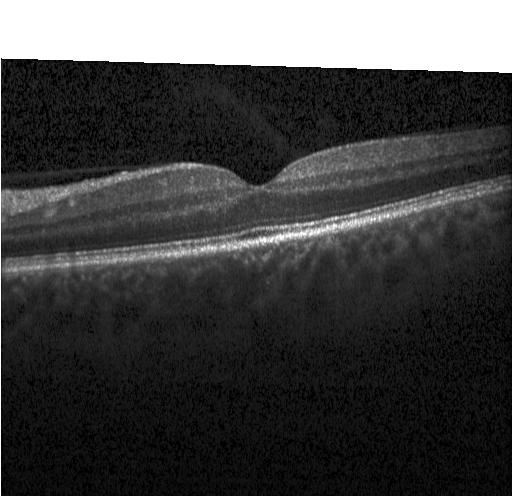

Spectral-domain OCT B-scan: no choroidal neovascularization, diabetic macular edema, or drusen.